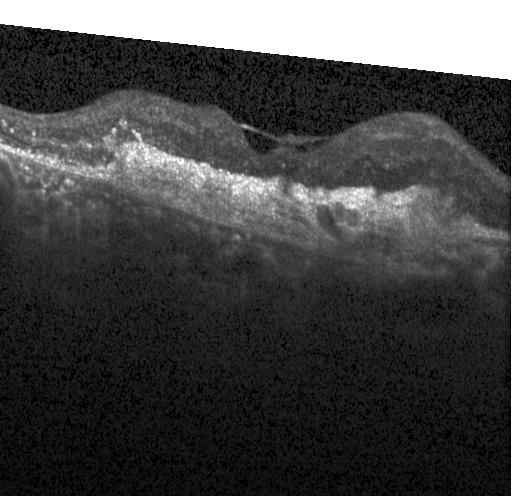 Impression: a choroidal neovascular membrane.